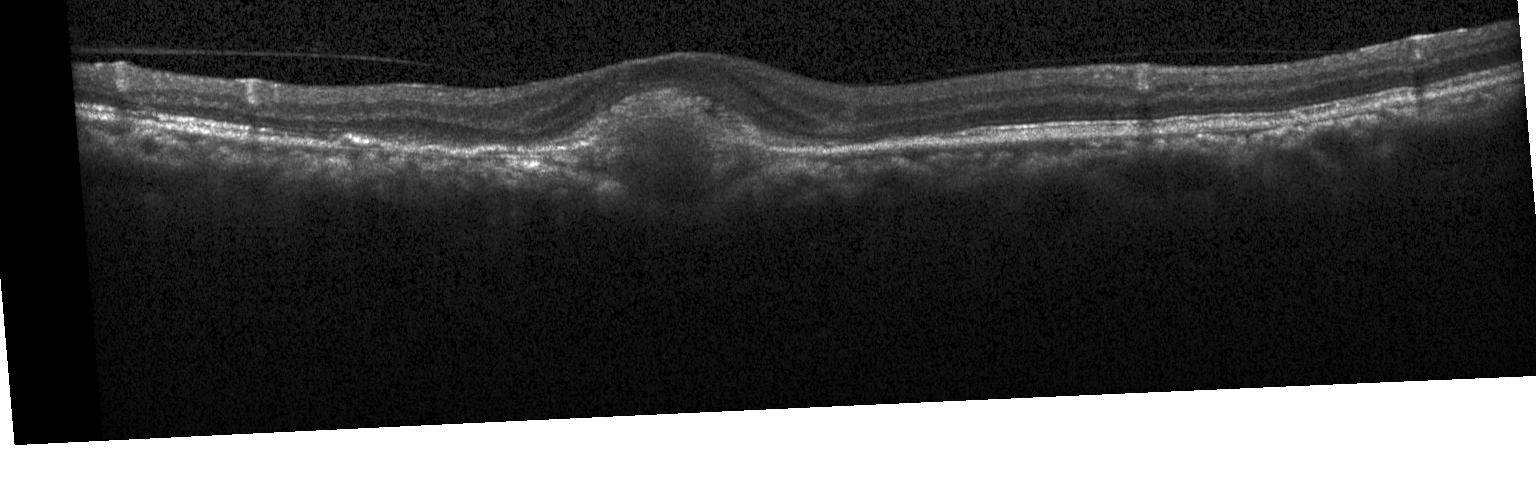

OCT finding: choroidal neovascularization.